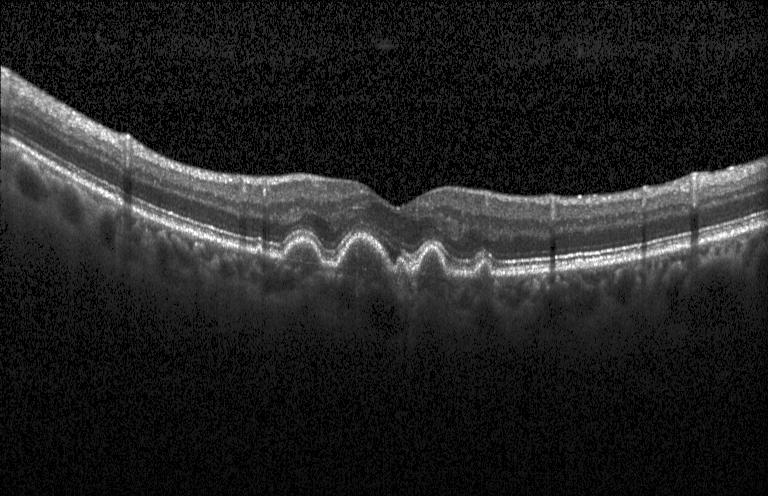
Impression: drusen.